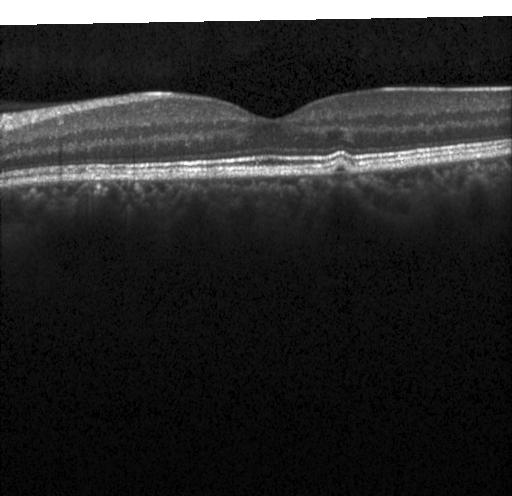 Finding: drusen.